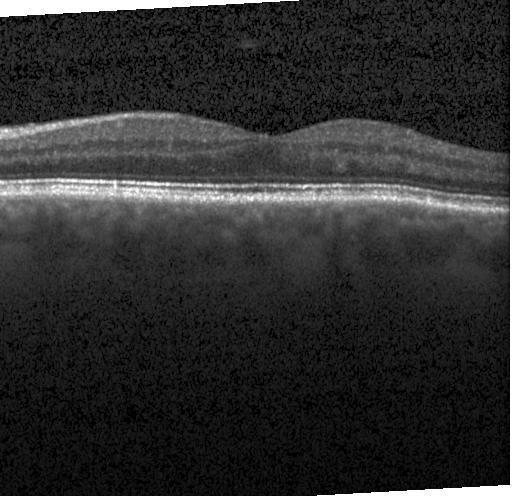
Macular OCT: no choroidal neovascularization, no diabetic macular edema, and no drusen.